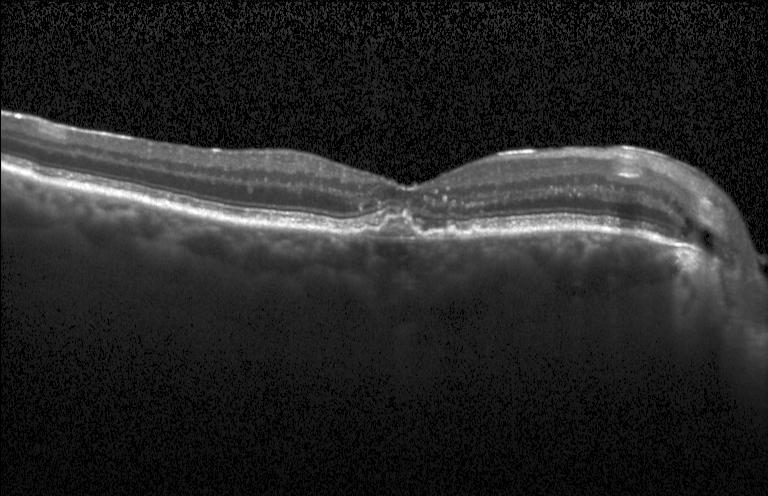
SD-OCT, instrument: Heidelberg Spectralis, optical coherence tomography B-scan — Macular OCT: CNV.